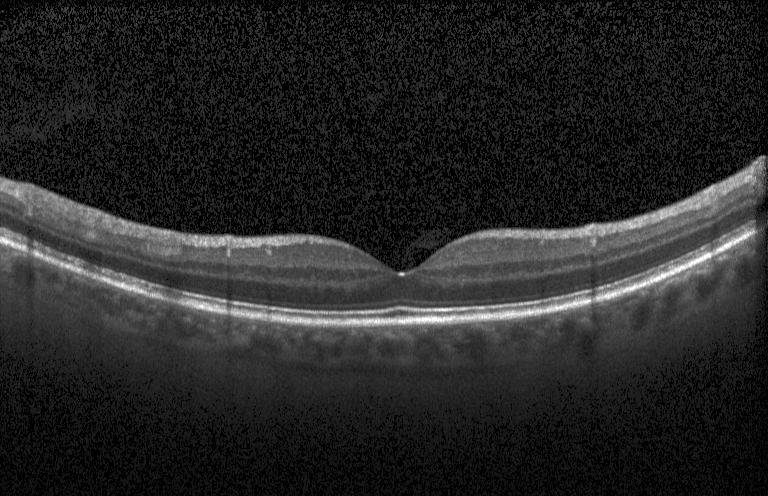 Dx: no choroidal neovascularization, diabetic macular edema, or drusen.